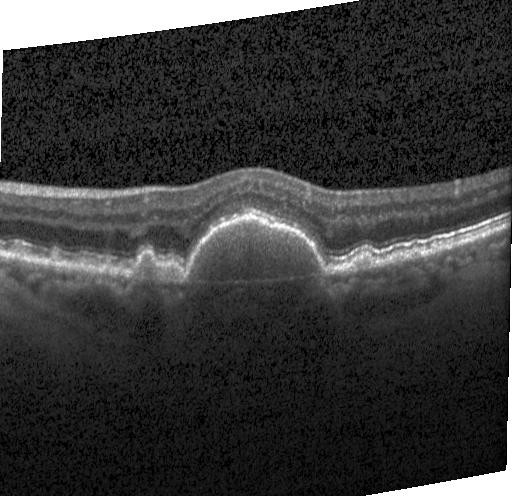 OCT line scan — Impression: choroidal neovascularization (CNV).